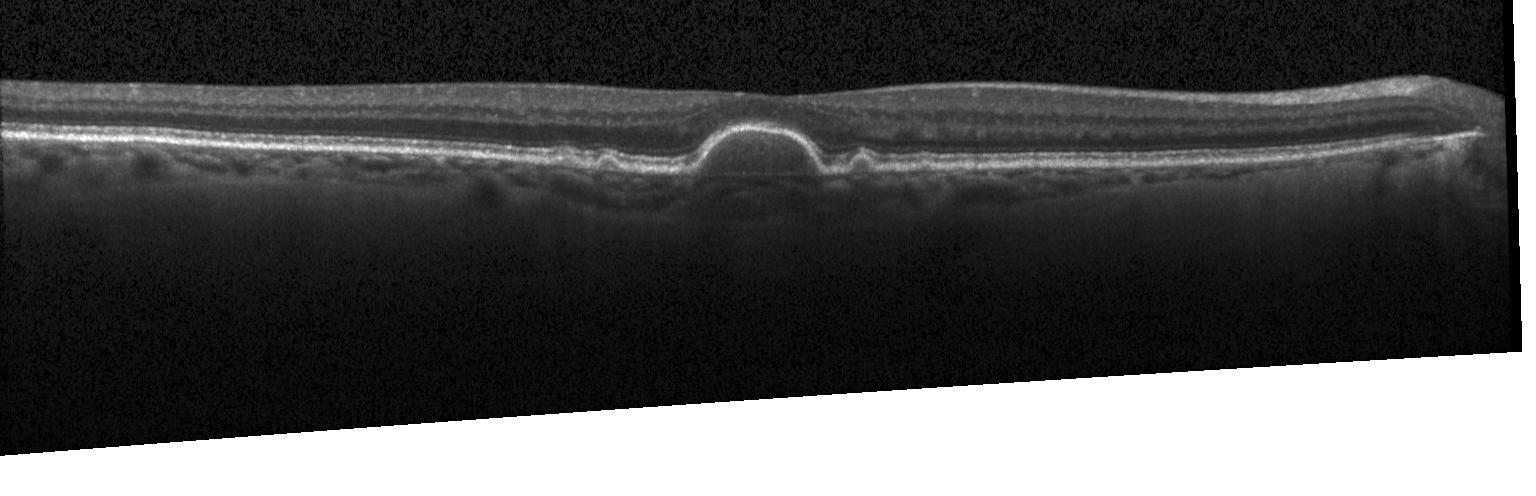

Retinal OCT cross-section
OCT finding: a choroidal neovascular membrane.